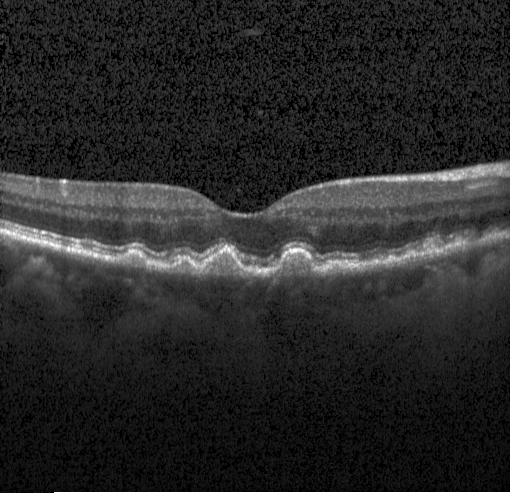 Retinal OCT B-scan; instrument: Heidelberg Spectralis
Diagnosis: sub-RPE drusenoid deposits.